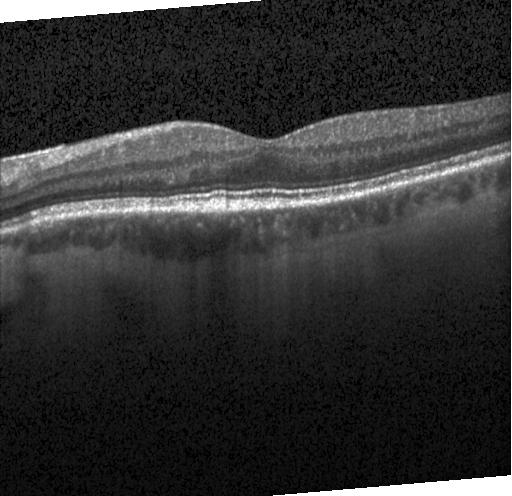

Retinal OCT cross-section. Neither choroidal neovascularization, diabetic macular edema, nor drusen.